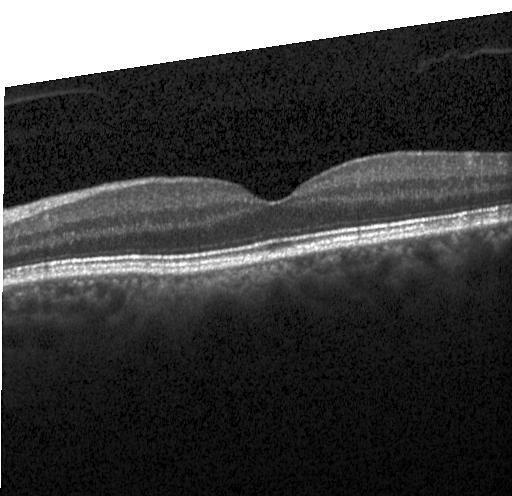

Acquired on a Heidelberg Spectralis, OCT line scan
Assessment: neither choroidal neovascularization, diabetic macular edema, nor drusen.